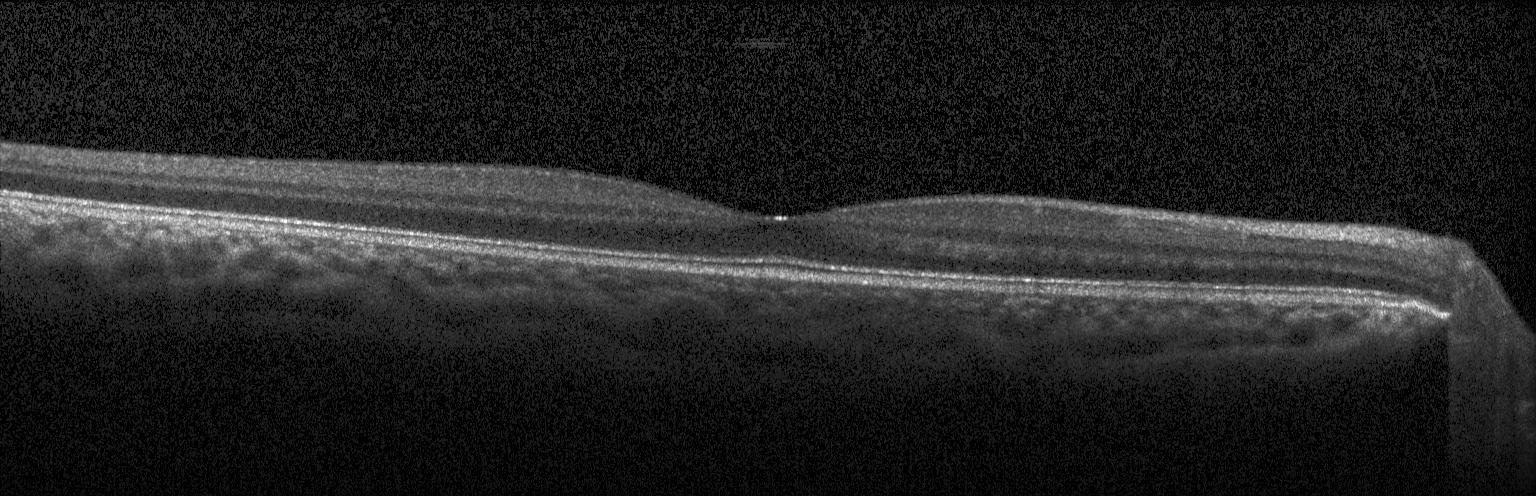 Impression: no evidence of choroidal neovascularization, diabetic macular edema, or drusen.